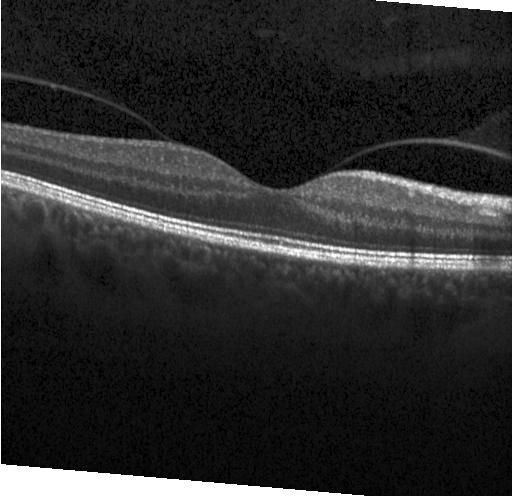 Spectral-domain optical coherence tomography. Retinal OCT cross-section. Heidelberg Spectralis.
Impression: no choroidal neovascularization, no diabetic macular edema, and no drusen.